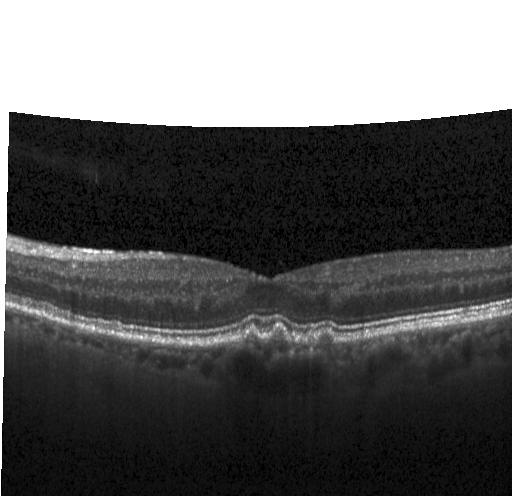
Macular OCT: drusen.